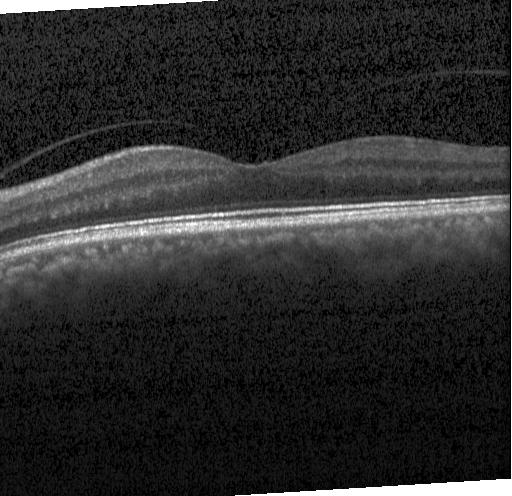
Finding: no choroidal neovascularization, no diabetic macular edema, and no drusen.